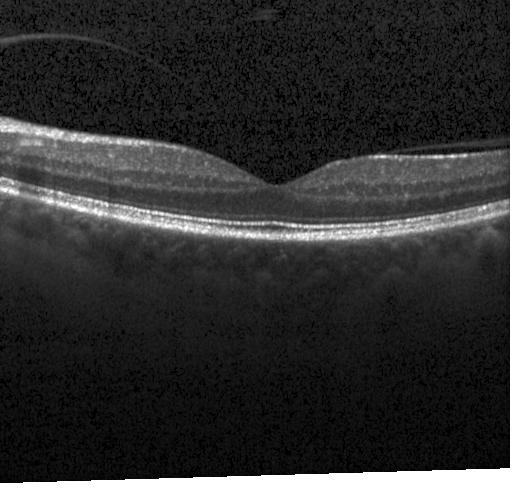
SD-OCT · horizontal scan through the fovea · instrument: Heidelberg Spectralis · OCT line scan.
Diagnosis: no evidence of choroidal neovascularization, diabetic macular edema, or drusen.